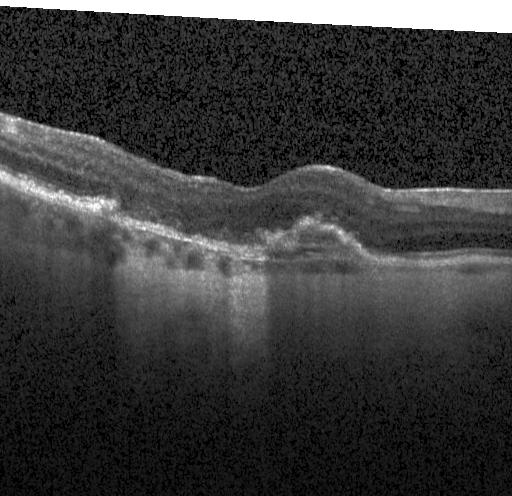

Impression: a choroidal neovascular membrane.